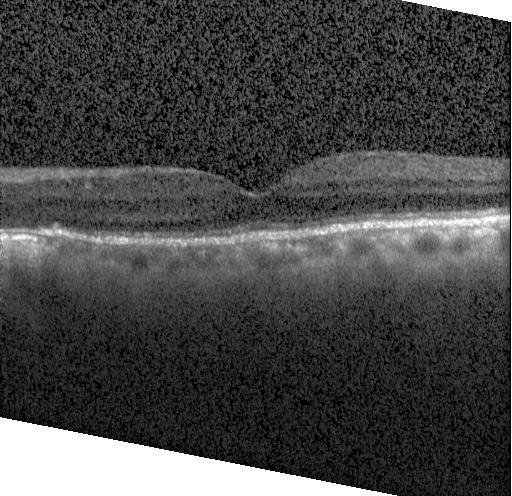 Spectral-domain OCT, instrument: Heidelberg Spectralis, optical coherence tomography scan, fovea-centered. Diagnosis: neither CNV, DME, nor drusen.